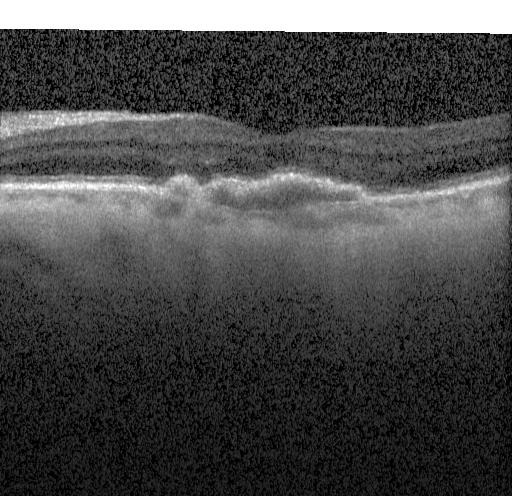 Optical coherence tomography B-scan. Horizontal scan through the fovea. Heidelberg Spectralis OCT system.
Diagnosis: a choroidal neovascular membrane.